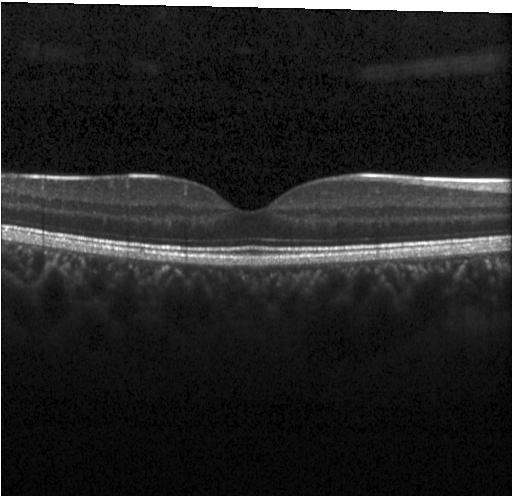 Diagnosis: no choroidal neovascularization, no diabetic macular edema, and no drusen.